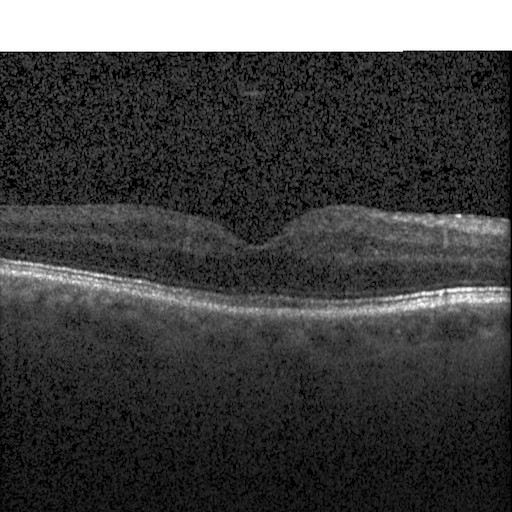 Macular OCT demonstrating diabetic macular edema.